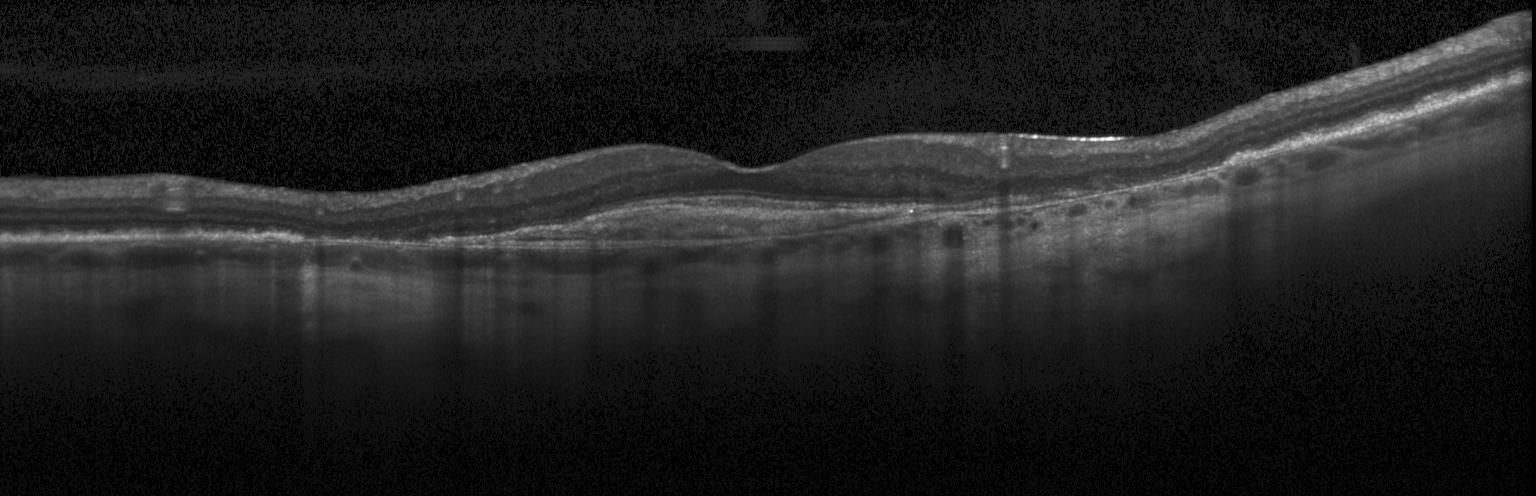

Retinal OCT B-scan. Spectral-domain OCT. Acquired on a Heidelberg Spectralis
Finding: choroidal neovascularization.